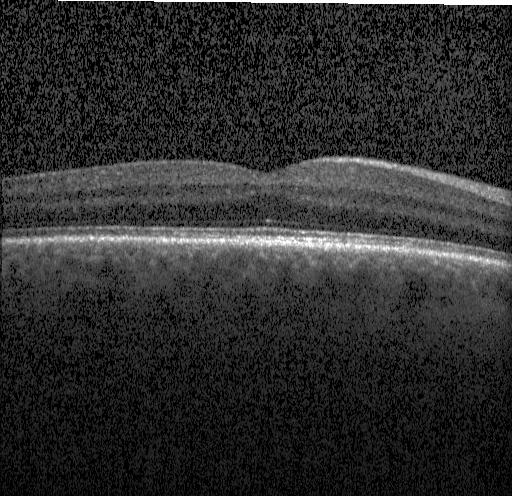

SD-OCT · Heidelberg Spectralis · through the macula · OCT line scan. Diagnosis: no evidence of choroidal neovascularization, diabetic macular edema, or drusen.